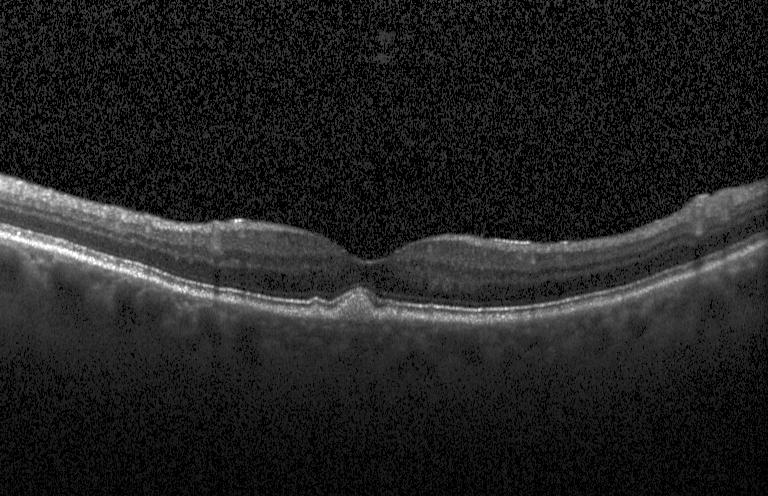
SD-OCT. Optical coherence tomography B-scan. Acquired on a Heidelberg Spectralis. Fovea-centered — Impression: drusen.